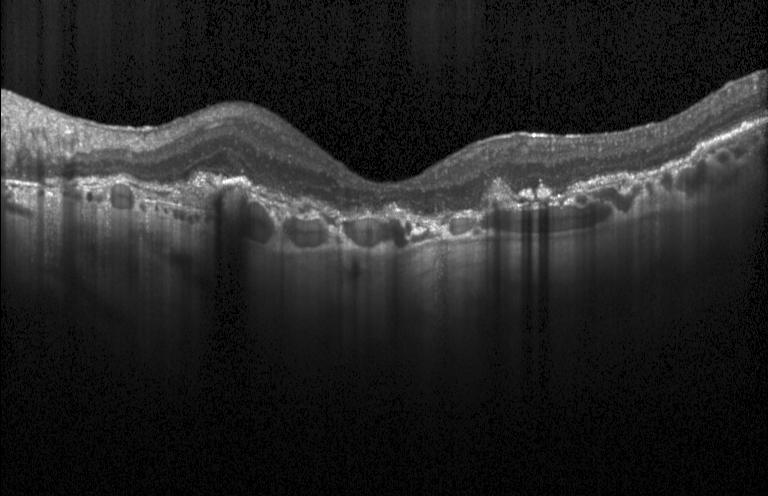 Diagnosis: CNV.